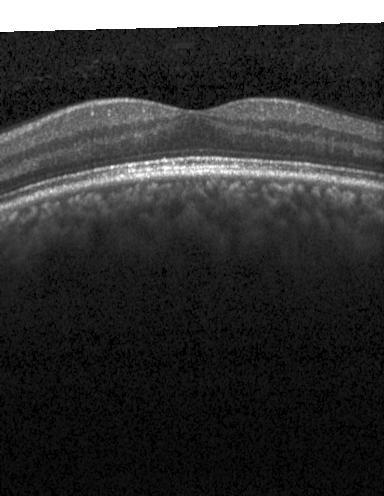

OCT line scan
Finding: no evidence of choroidal neovascularization, diabetic macular edema, or drusen.